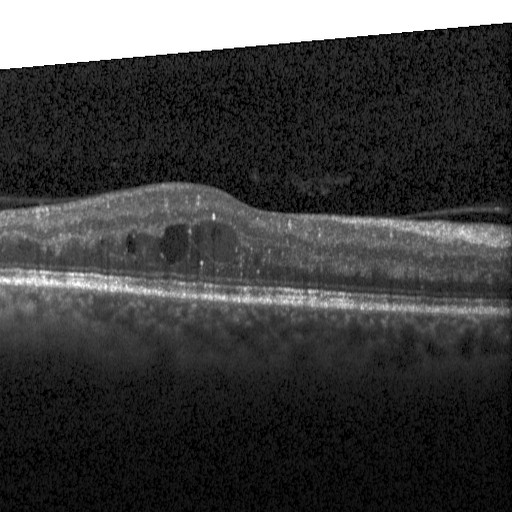
Fovea-centered · Heidelberg Spectralis · spectral-domain optical coherence tomography · optical coherence tomography B-scan.
Impression: DME.